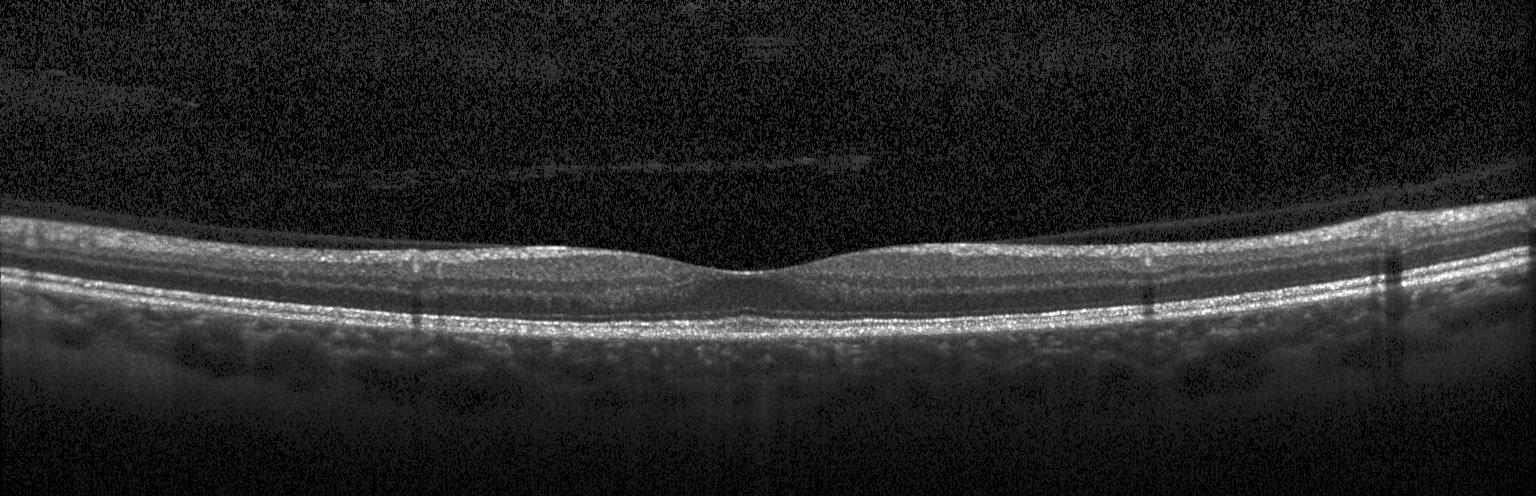 Optical coherence tomography scan, fovea-centered — Finding: neither choroidal neovascularization, diabetic macular edema, nor drusen.